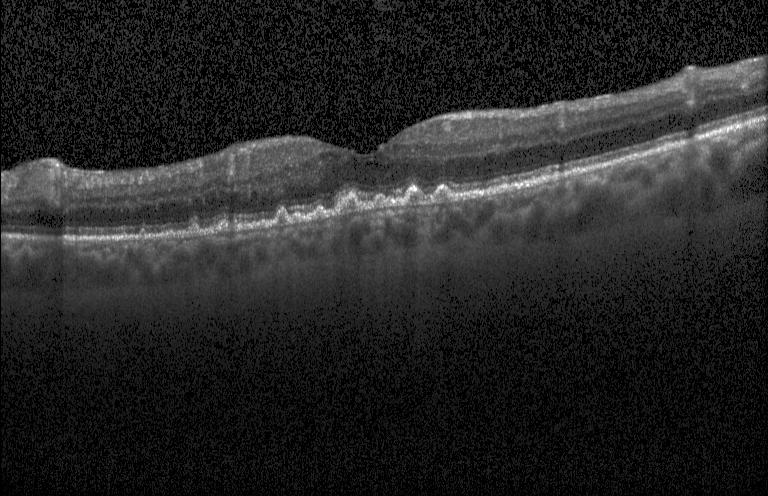 Retinal OCT cross-section showing sub-RPE drusenoid deposits.